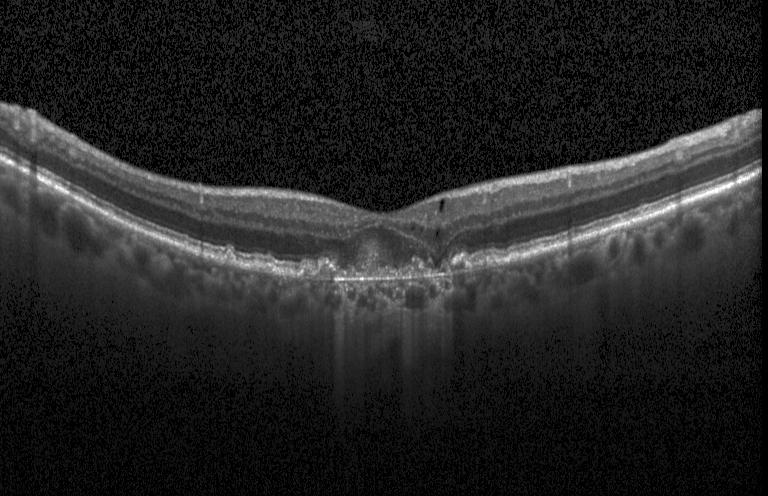
Retinal OCT B-scan — Diagnosis: choroidal neovascularization (CNV).